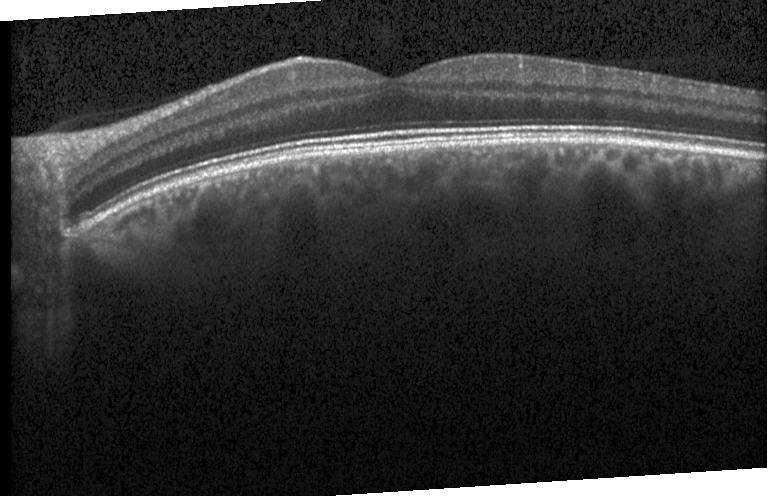 Dx: no evidence of choroidal neovascularization, diabetic macular edema, or drusen.